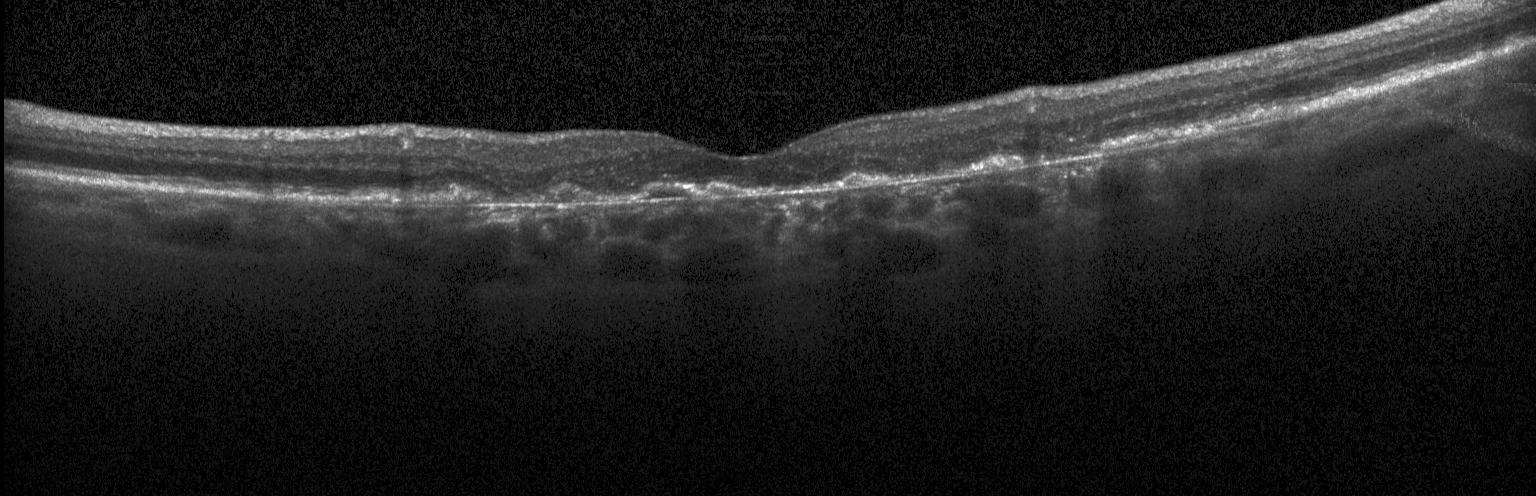

Assessment: choroidal neovascularization.